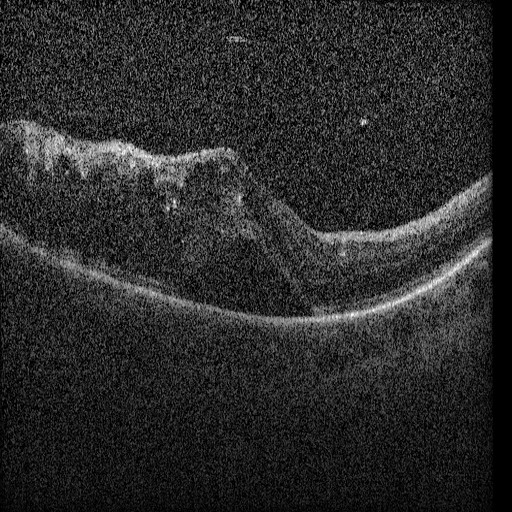 OCT B-scan showing diabetic macular edema.